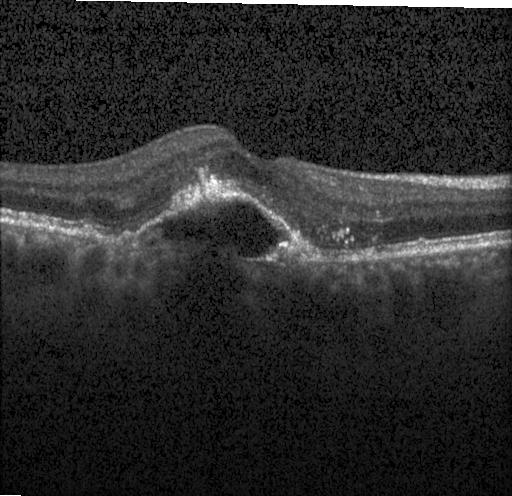

Retinal OCT cross-section. Diagnosis: a choroidal neovascular membrane.